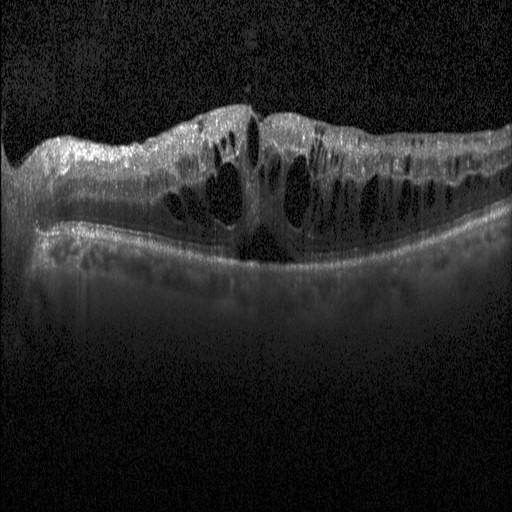
Instrument: Heidelberg Spectralis; fovea-centered; optical coherence tomography scan; spectral-domain OCT. Diagnosis: diabetic macular edema (DME).